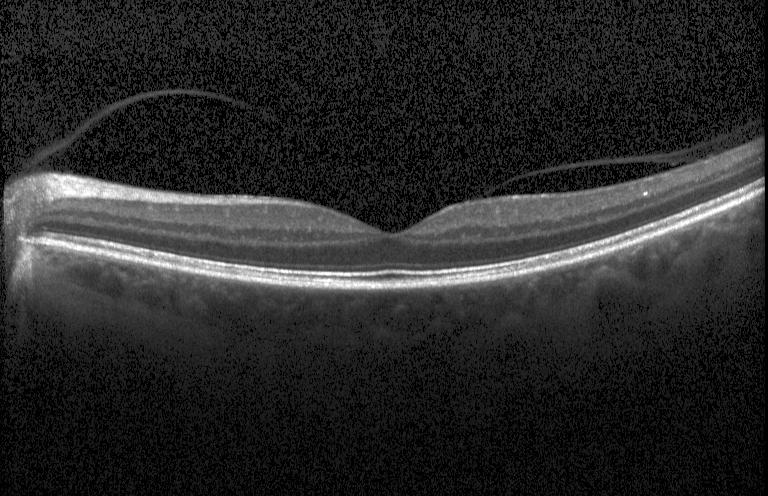

Retinal OCT B-scan
This B-scan demonstrates neither choroidal neovascularization, diabetic macular edema, nor drusen.